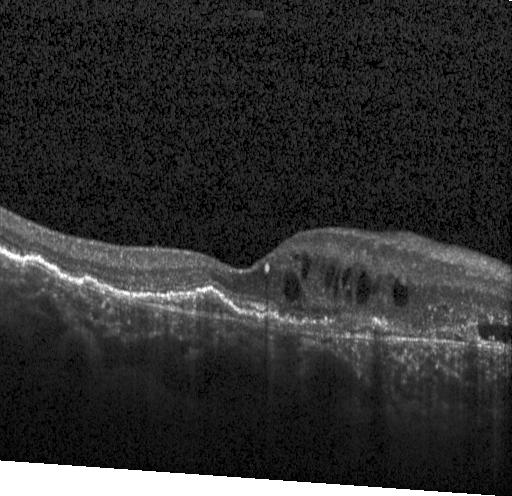
Retinal OCT cross-section showing a choroidal neovascular membrane.